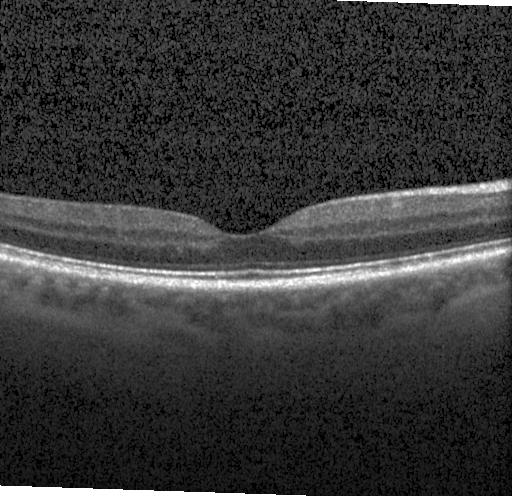 Assessment: neither choroidal neovascularization, diabetic macular edema, nor drusen.